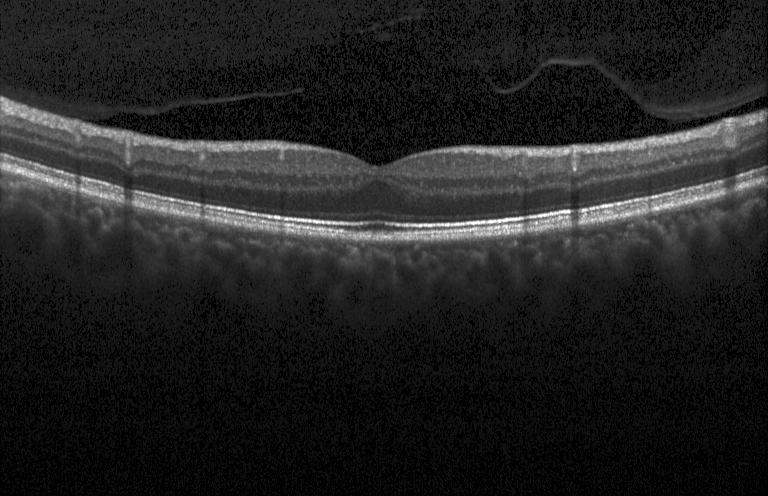 Finding: neither CNV, DME, nor drusen.